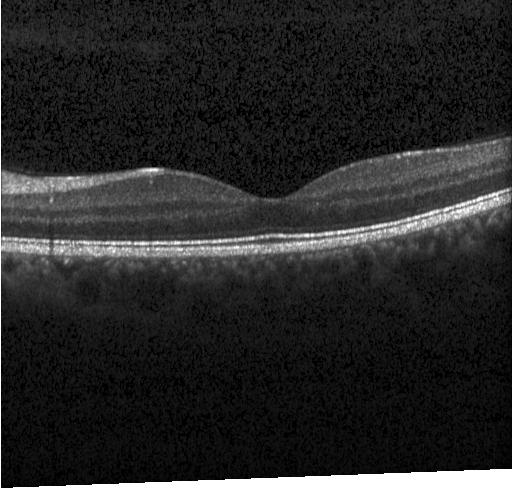

OCT B-scan
Macular OCT: no CNV, DME, or drusen.